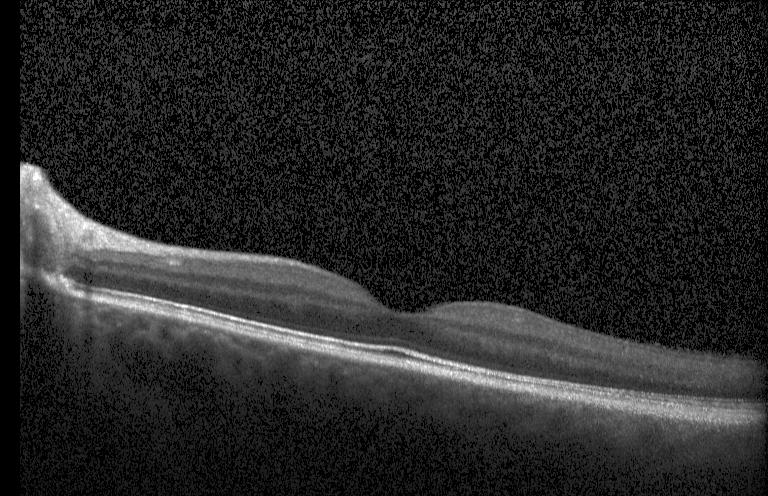

OCT line scan. OCT finding: no choroidal neovascularization, diabetic macular edema, or drusen.